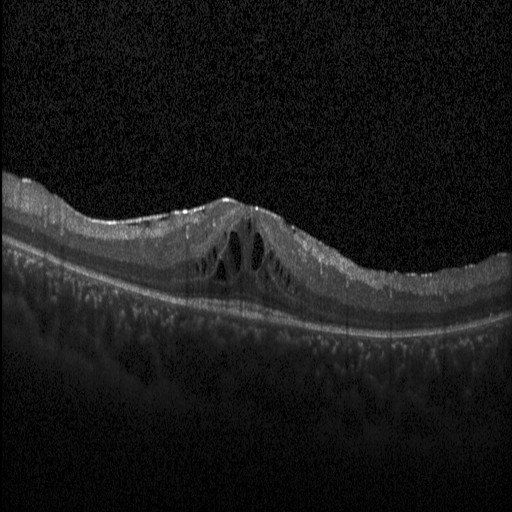
Assessment: DME.